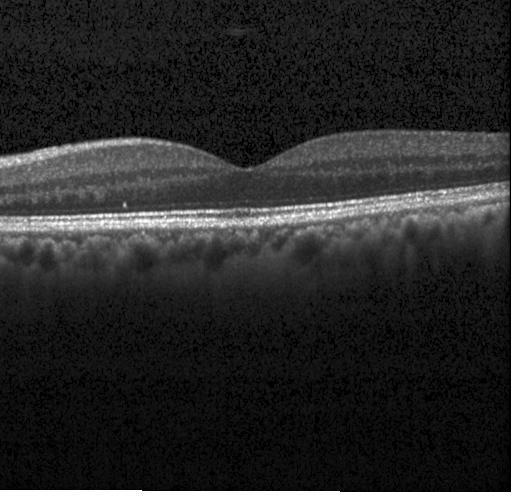

Heidelberg Spectralis, OCT line scan, spectral-domain OCT
Impression: neither CNV, DME, nor drusen.